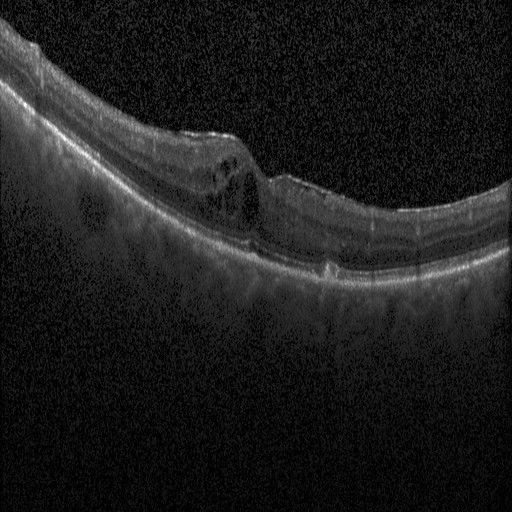 Diagnosis: diabetic macular edema.